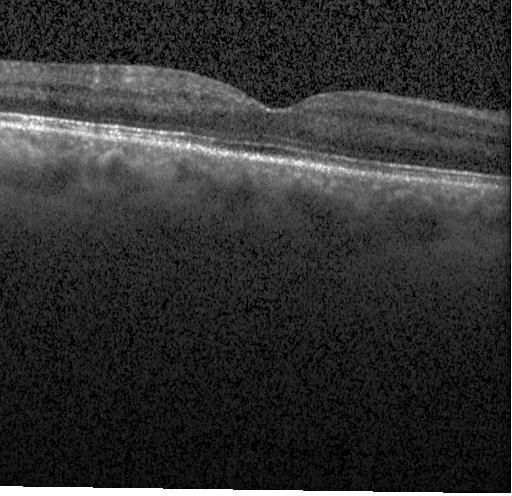

Retinal OCT B-scan. Spectral-domain optical coherence tomography.
This B-scan demonstrates no CNV, no DME, and no drusen.